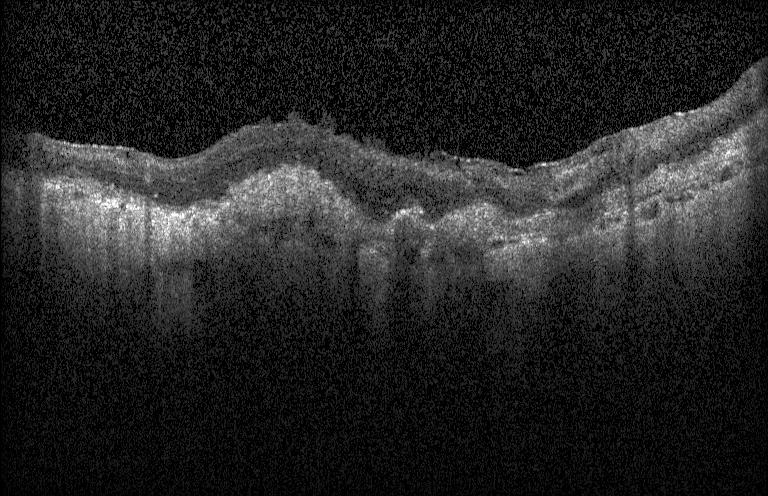

Assessment: choroidal neovascularization.